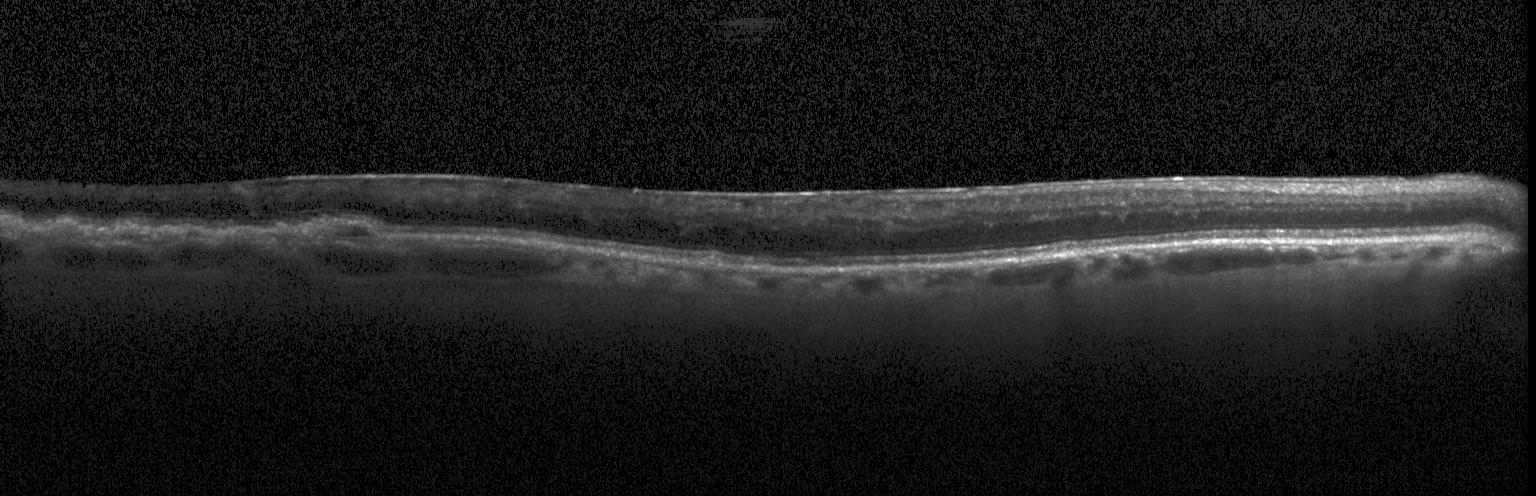

Finding: a choroidal neovascular membrane.